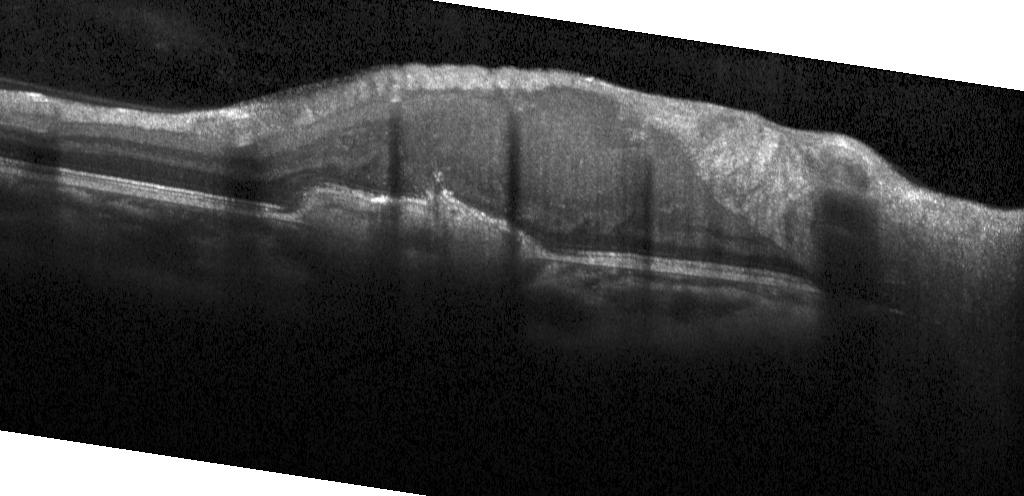
Macular OCT demonstrating choroidal neovascularization.